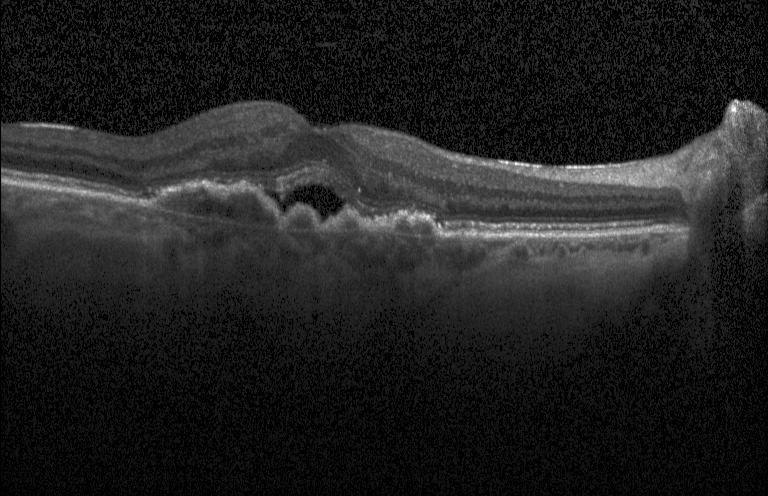

Acquired on a Heidelberg Spectralis; spectral-domain optical coherence tomography; optical coherence tomography scan; centered on the fovea.
Finding: CNV.